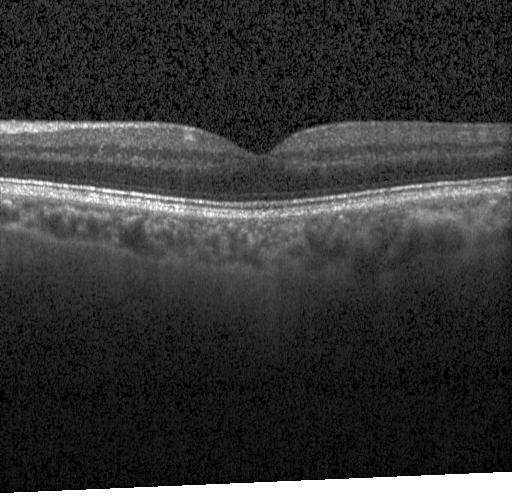 Horizontal scan through the fovea; acquired on a Heidelberg Spectralis; optical coherence tomography scan. Assessment: no CNV, no DME, and no drusen.